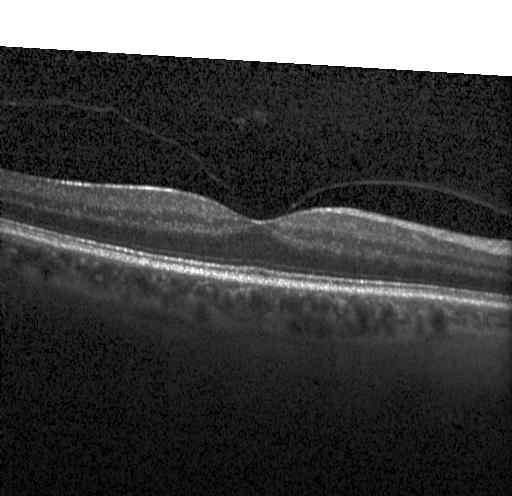

OCT B-scan showing no CNV, DME, or drusen.